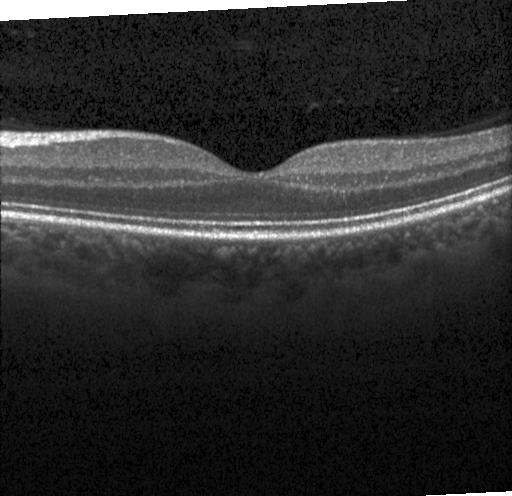 OCT B-scan showing no evidence of choroidal neovascularization, diabetic macular edema, or drusen.